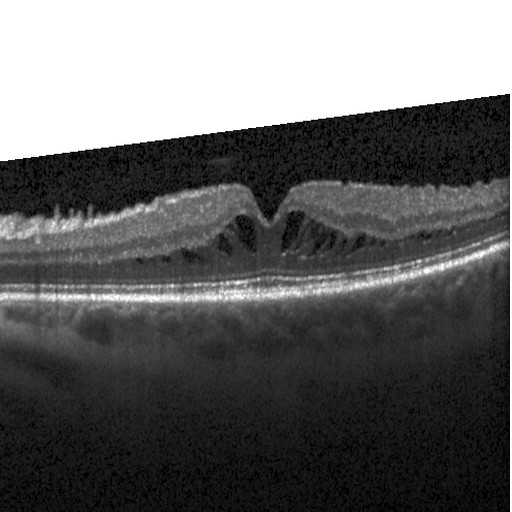
Retinal OCT cross-section.
DME.